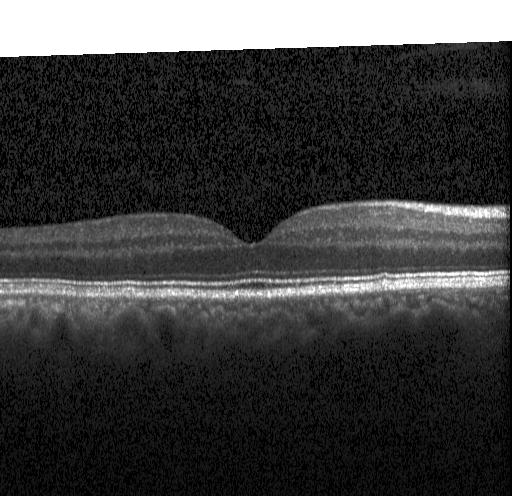
Retinal OCT cross-section showing no evidence of CNV, DME, or drusen.